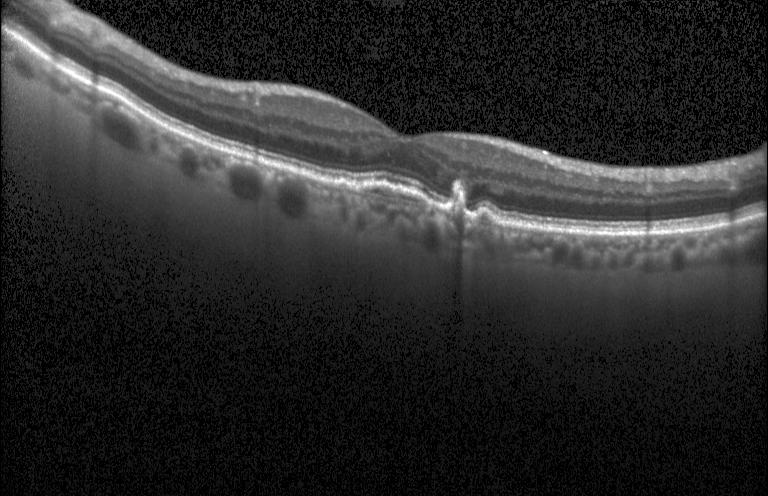

Horizontal scan through the fovea; optical coherence tomography B-scan; acquired on a Heidelberg Spectralis; spectral-domain OCT
The scan shows a choroidal neovascular membrane.